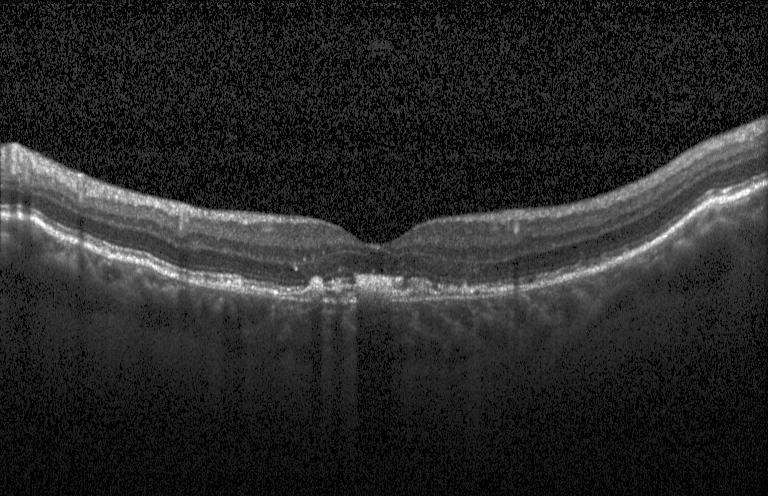

Fovea-centered; optical coherence tomography scan; spectral-domain OCT.
Dx: a choroidal neovascular membrane.